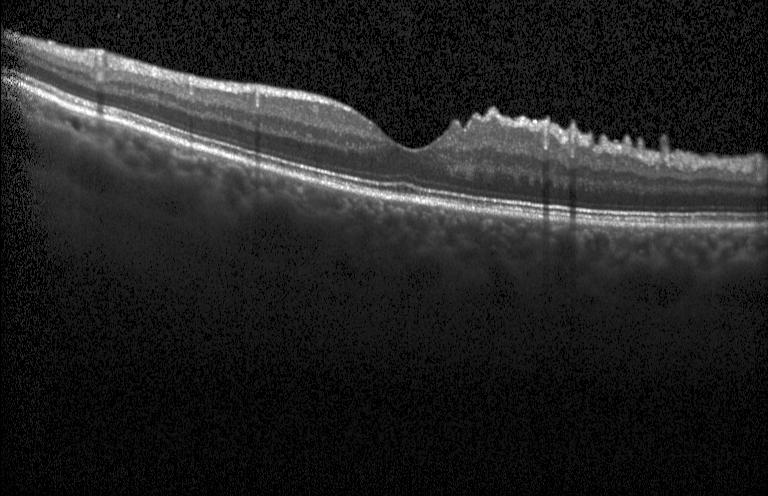

Optical coherence tomography B-scan — The scan shows no CNV, no DME, and no drusen.